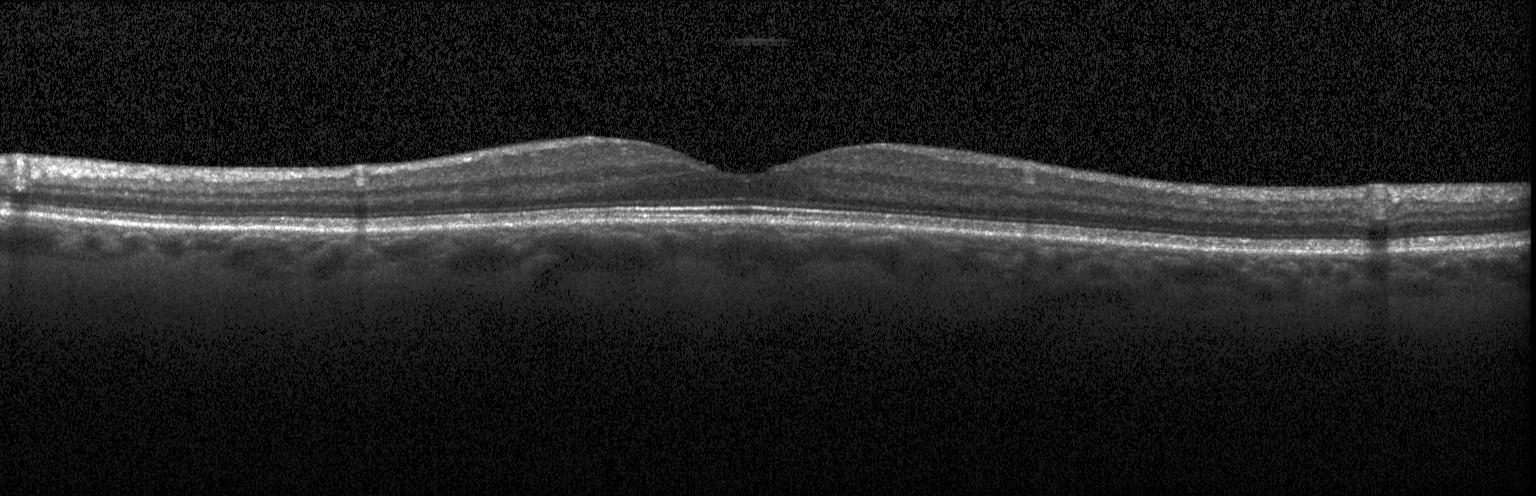

Optical coherence tomography B-scan. Finding: no evidence of choroidal neovascularization, diabetic macular edema, or drusen.